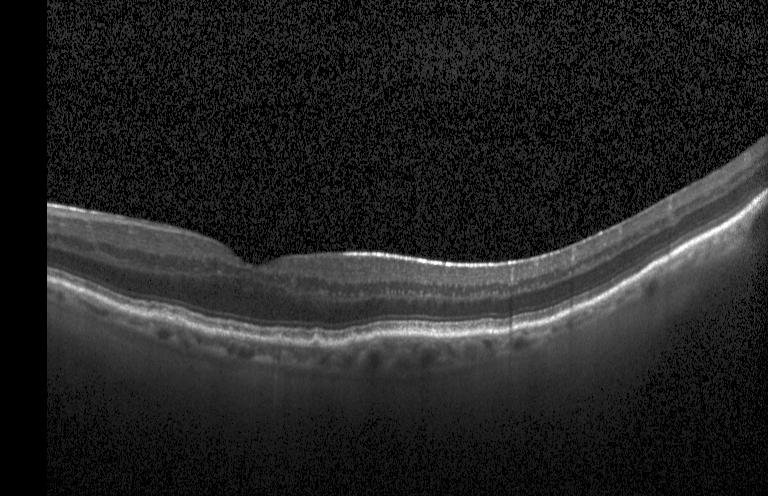

Fovea-centered, Heidelberg Spectralis OCT system, OCT B-scan
This B-scan demonstrates sub-RPE drusenoid deposits.